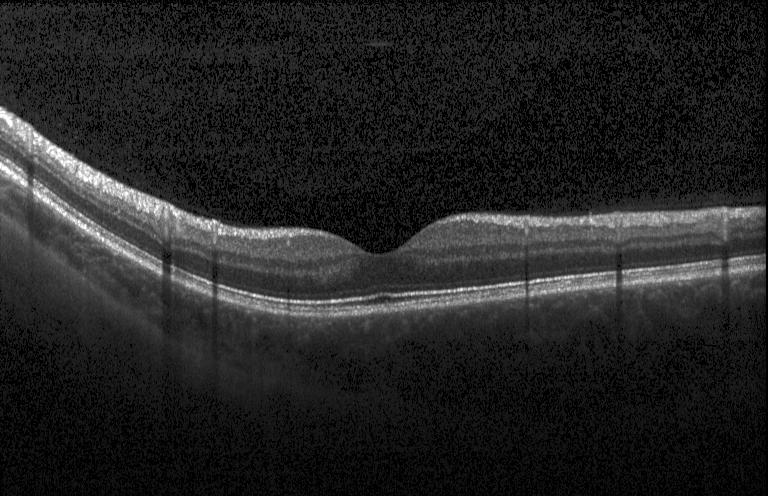
Optical coherence tomography scan. Dx: no CNV, DME, or drusen.